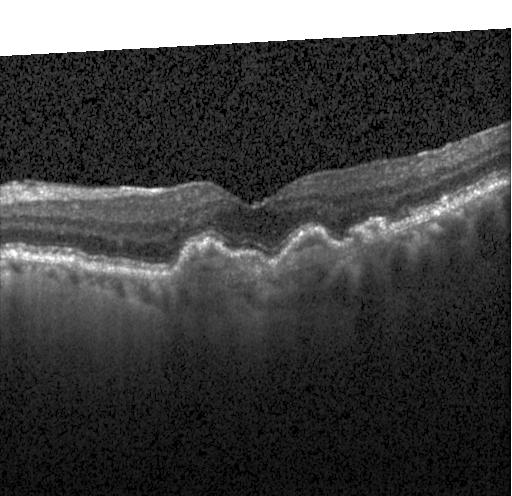
OCT finding: choroidal neovascularization (CNV).